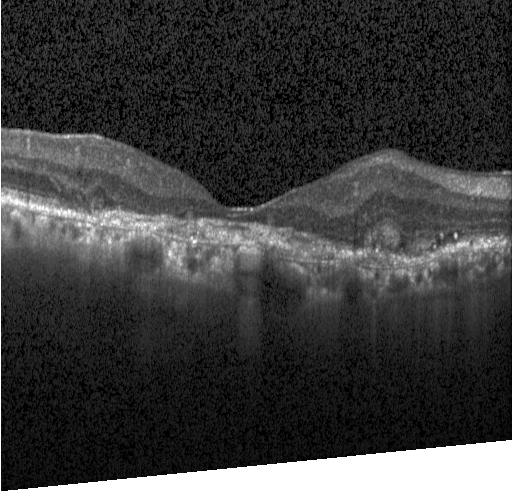 Spectral-domain optical coherence tomography. Heidelberg Spectralis OCT system. OCT B-scan. Macular scan.
The scan shows a choroidal neovascular membrane.